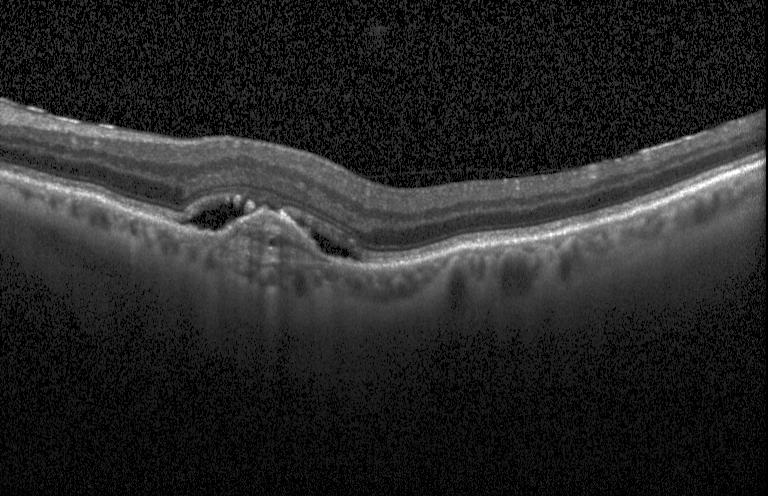 OCT finding: a choroidal neovascular membrane.